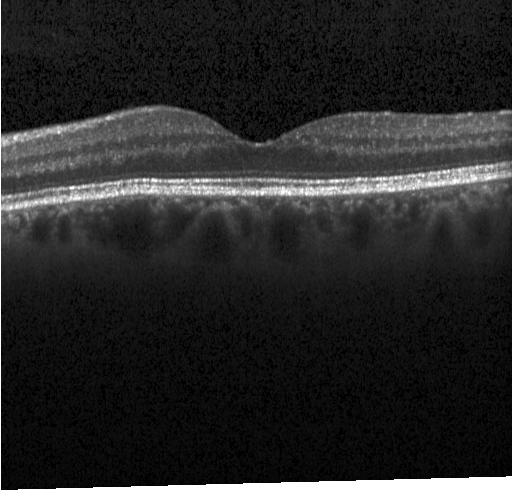 Diagnosis: neither choroidal neovascularization, diabetic macular edema, nor drusen.